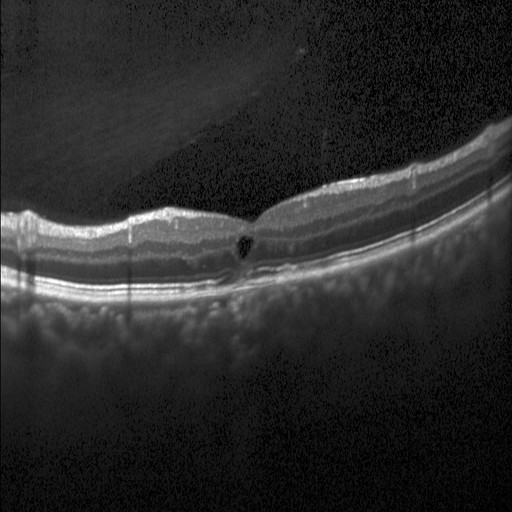

OCT B-scan; Heidelberg Spectralis. Dx: diabetic macular edema (DME).